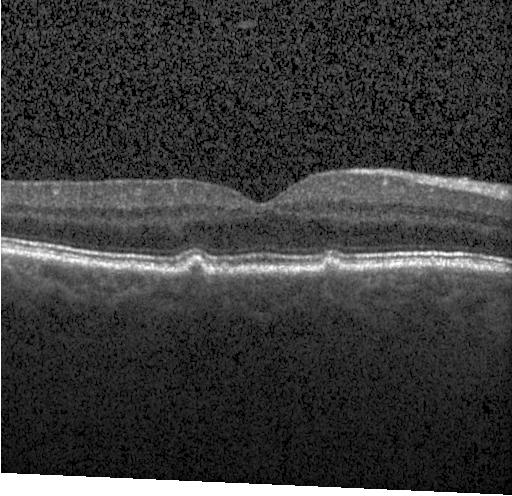

Heidelberg Spectralis. Optical coherence tomography B-scan. Horizontal scan through the fovea. Spectral-domain optical coherence tomography. This B-scan demonstrates multiple drusen.